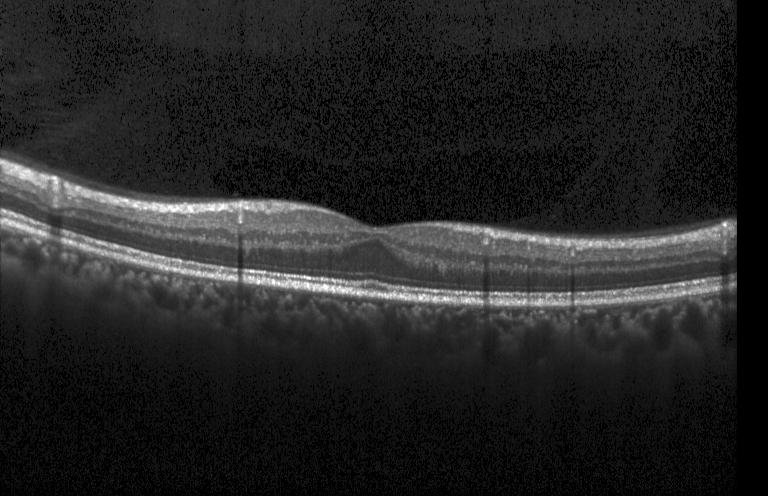

Assessment: no CNV, DME, or drusen.